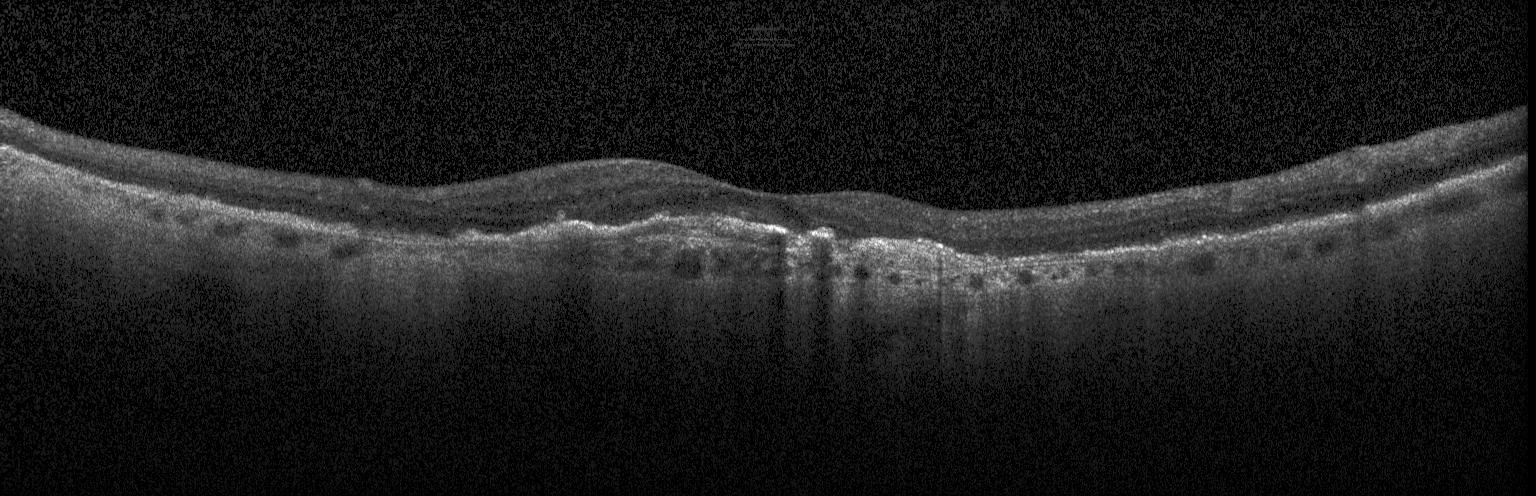
Retinal OCT cross-section.
Macular OCT: CNV.